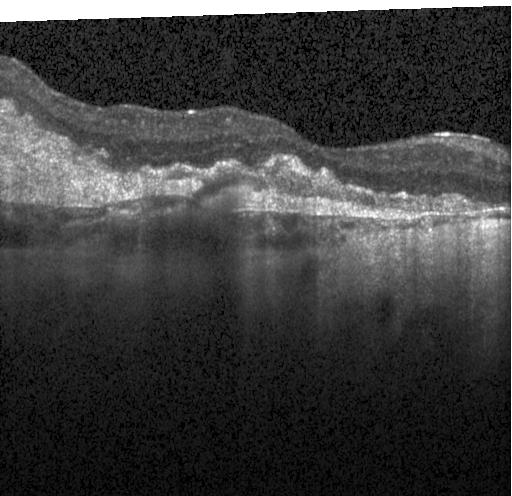

Retinal OCT B-scan · SD-OCT.
Macular OCT: a choroidal neovascular membrane.